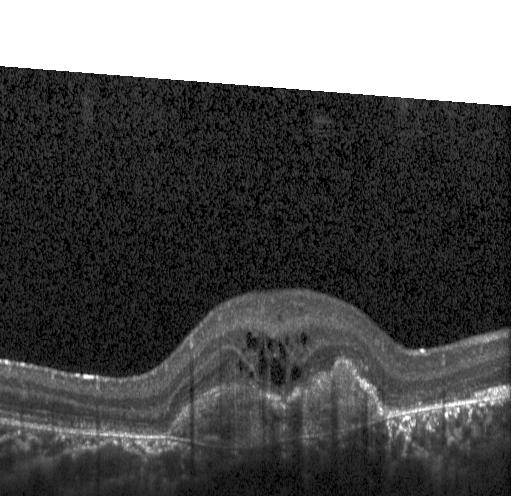

OCT B-scan. The scan shows a choroidal neovascular membrane.